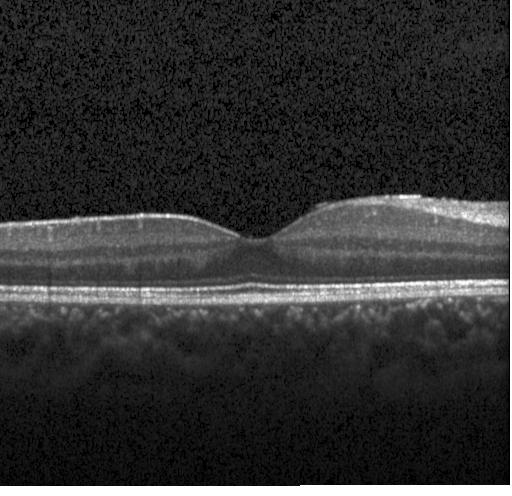

OCT line scan; Heidelberg Spectralis OCT system. No choroidal neovascularization, diabetic macular edema, or drusen.